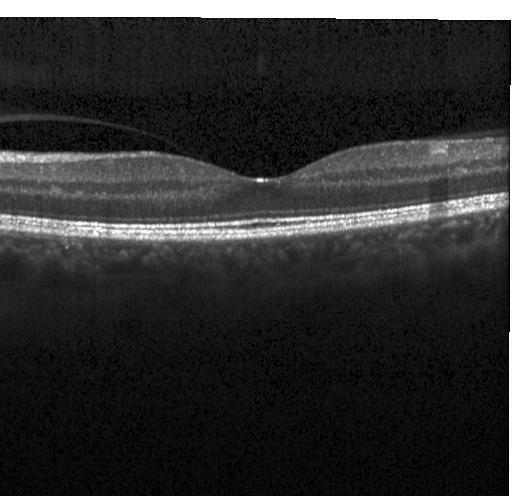
Retinal OCT B-scan; spectral-domain optical coherence tomography. This B-scan demonstrates no CNV, DME, or drusen.